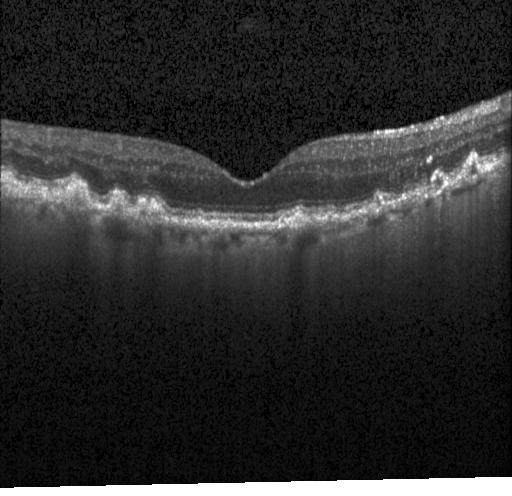

Heidelberg Spectralis OCT system; retinal OCT B-scan; SD-OCT; macular scan.
Impression: sub-RPE drusenoid deposits.